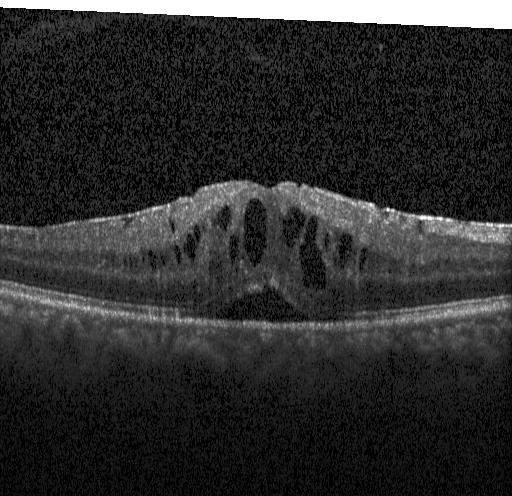
OCT line scan · instrument: Heidelberg Spectralis · fovea-centered — Assessment: diabetic macular edema.